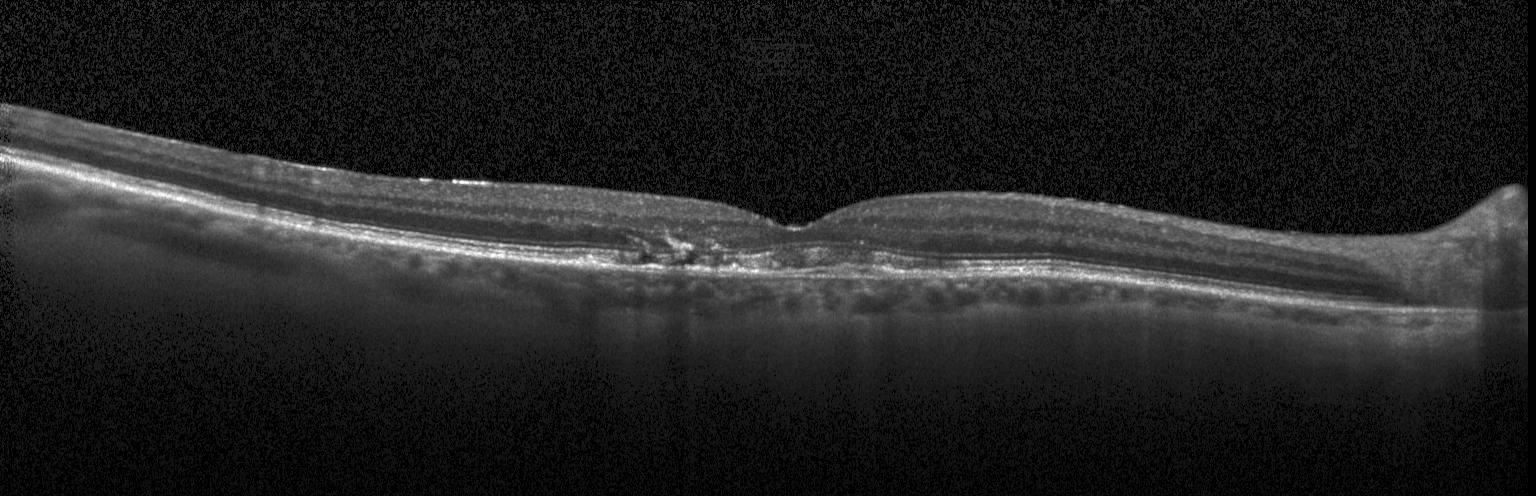 CNV.